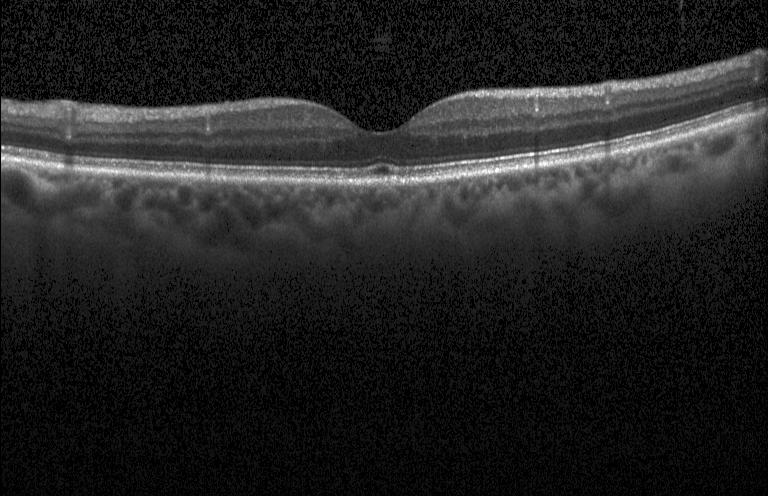 Spectral-domain OCT, OCT B-scan, Heidelberg Spectralis OCT system, centered on the fovea
No choroidal neovascularization, diabetic macular edema, or drusen.